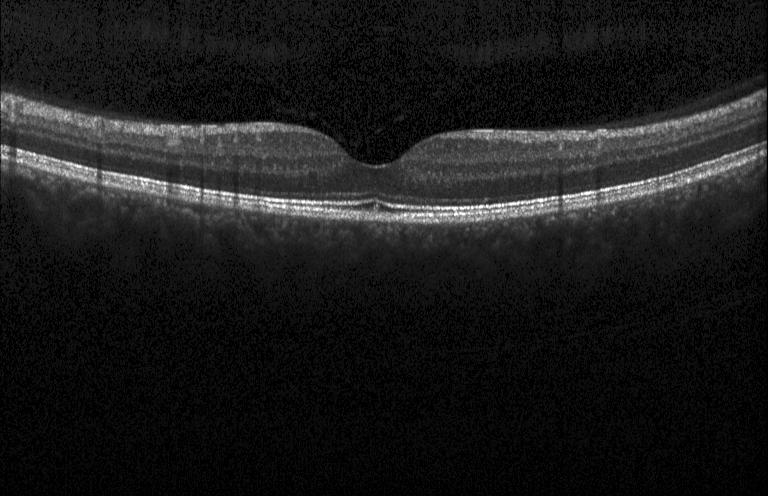

Centered on the fovea. Instrument: Heidelberg Spectralis. SD-OCT. OCT line scan. Diagnosis: no CNV, no DME, and no drusen.